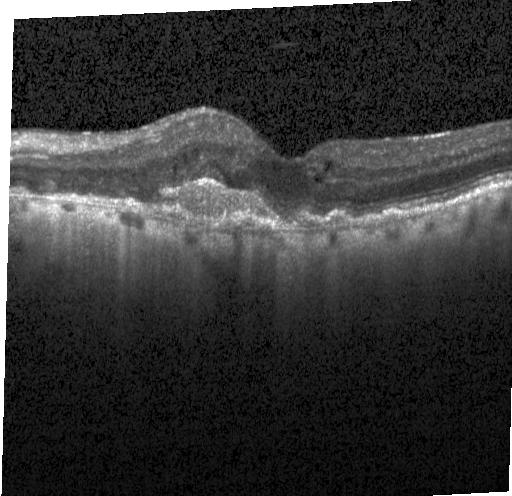 Optical coherence tomography B-scan; spectral-domain optical coherence tomography — This B-scan demonstrates choroidal neovascularization (CNV).